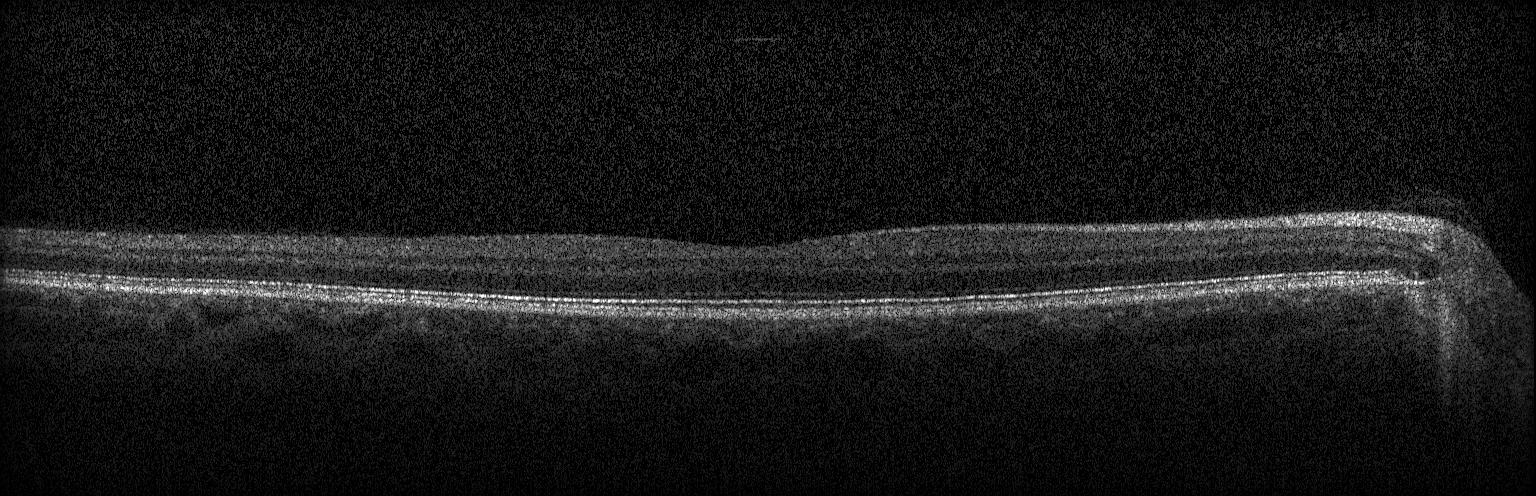
Retinal OCT B-scan, Heidelberg Spectralis OCT system, SD-OCT. Diagnosis: neither choroidal neovascularization, diabetic macular edema, nor drusen.